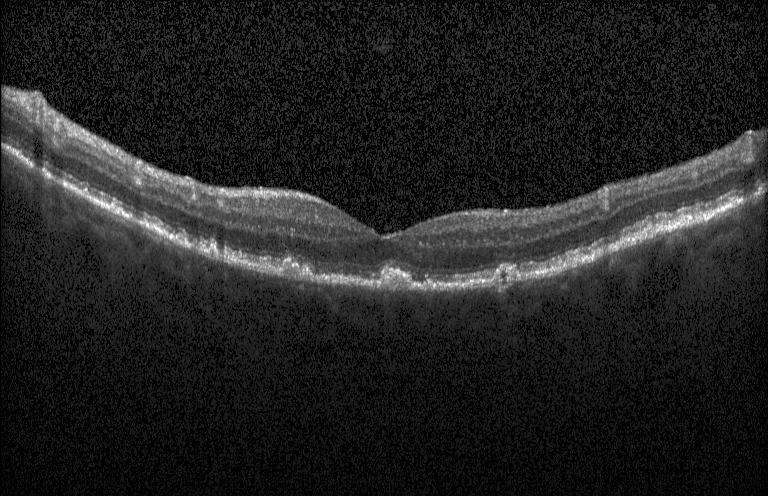
Retinal OCT cross-section showing CNV.